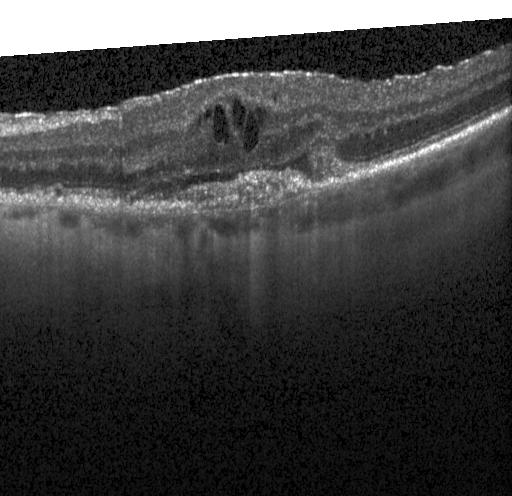 Retinal OCT cross-section
Choroidal neovascularization (CNV).